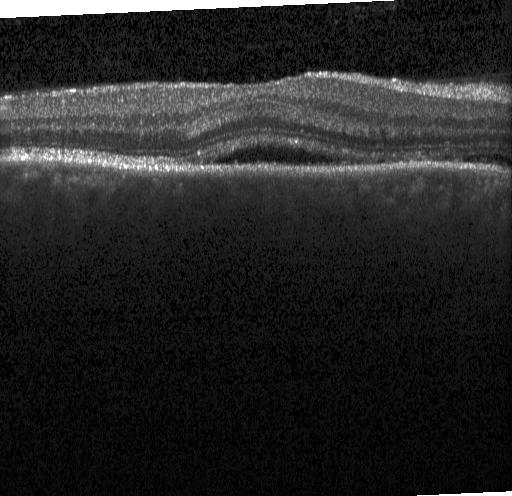

Finding: a choroidal neovascular membrane.